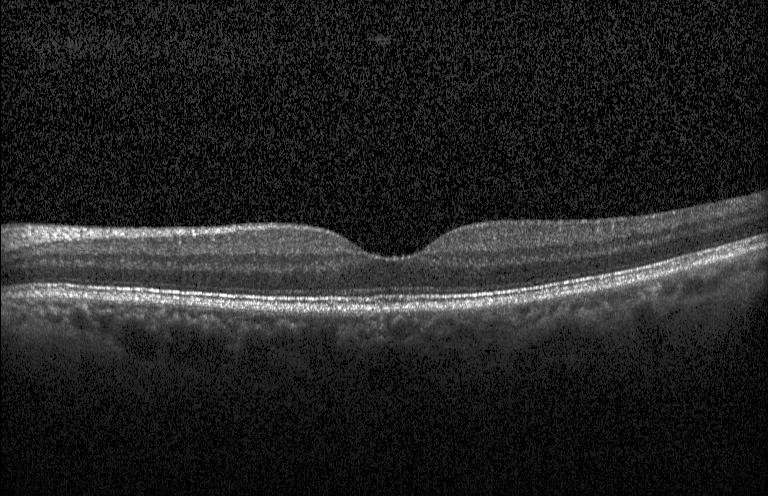

Finding: no choroidal neovascularization, no diabetic macular edema, and no drusen.